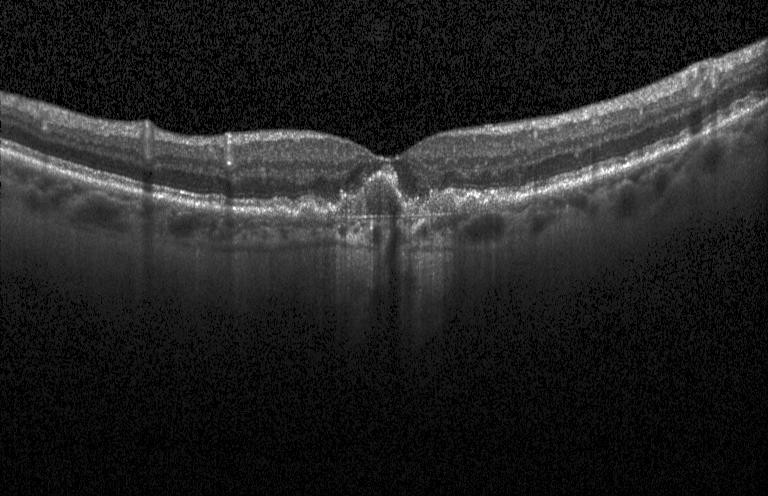 OCT line scan — Impression: a choroidal neovascular membrane.